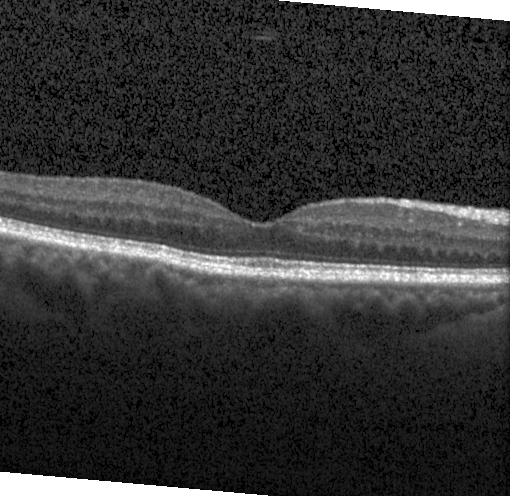
Neither choroidal neovascularization, diabetic macular edema, nor drusen.